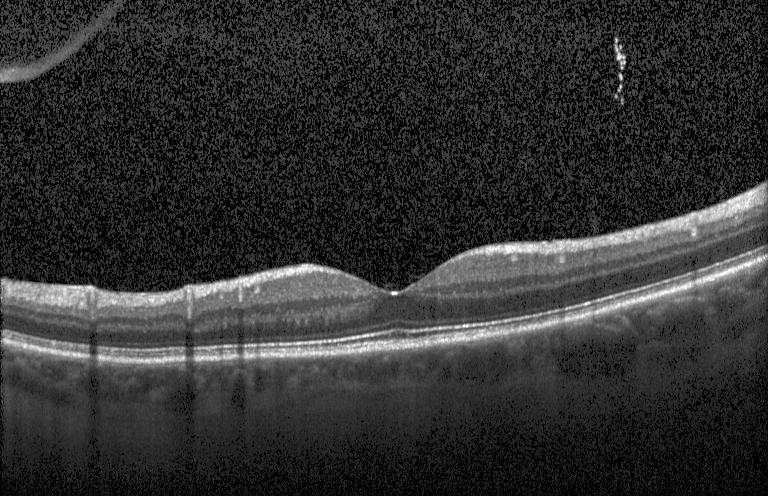
OCT line scan — Impression: no choroidal neovascularization, diabetic macular edema, or drusen.